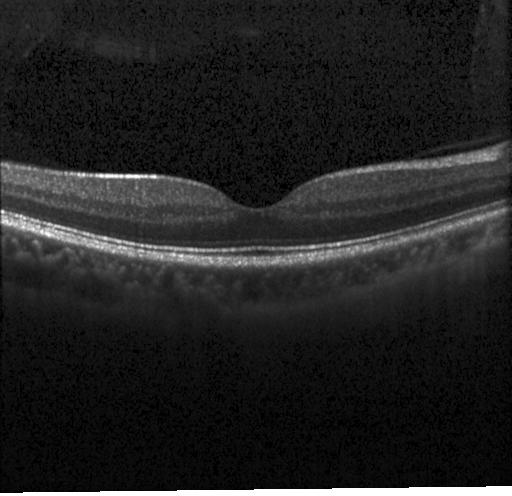
Macular OCT demonstrating no choroidal neovascularization, no diabetic macular edema, and no drusen.